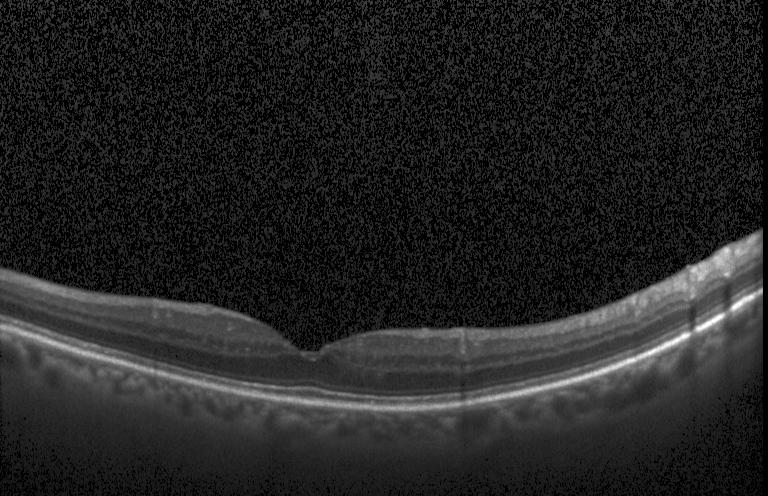

The scan shows neither choroidal neovascularization, diabetic macular edema, nor drusen.